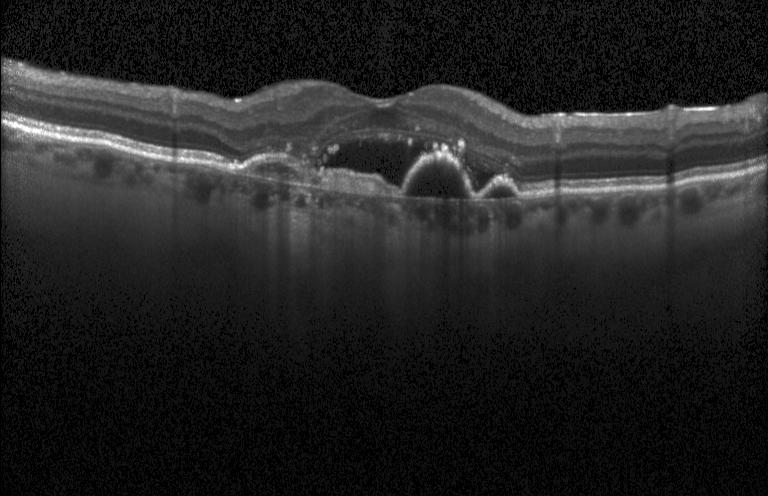 Retinal OCT B-scan — Macular OCT: a choroidal neovascular membrane.